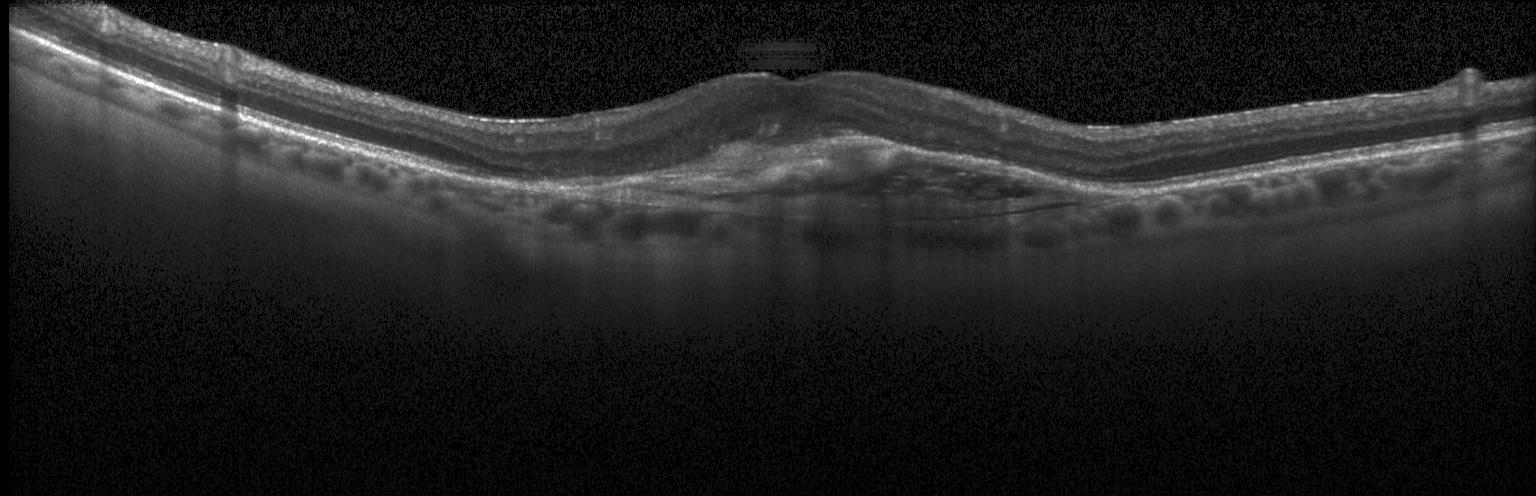 Macular OCT demonstrating a choroidal neovascular membrane.